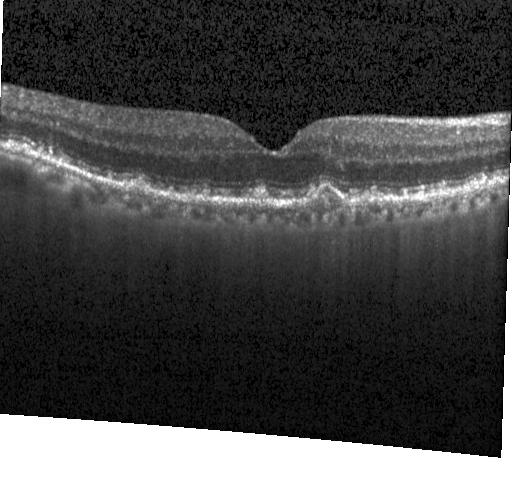

OCT line scan
Finding: sub-RPE drusenoid deposits.